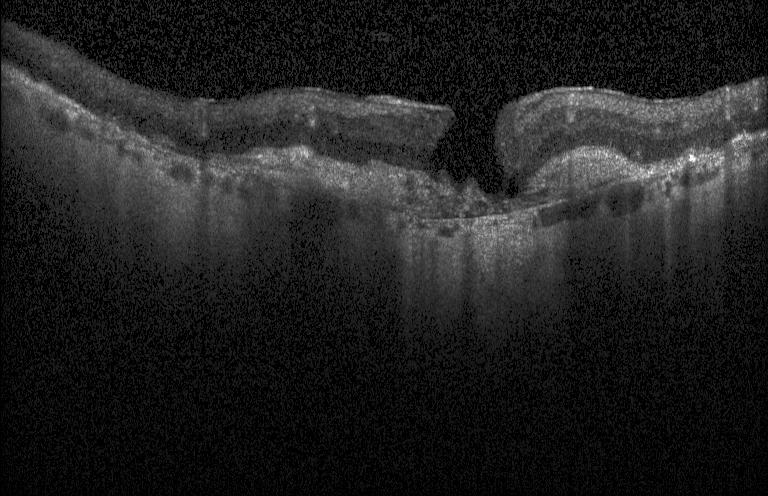
Retinal OCT cross-section, SD-OCT — Impression: a choroidal neovascular membrane.